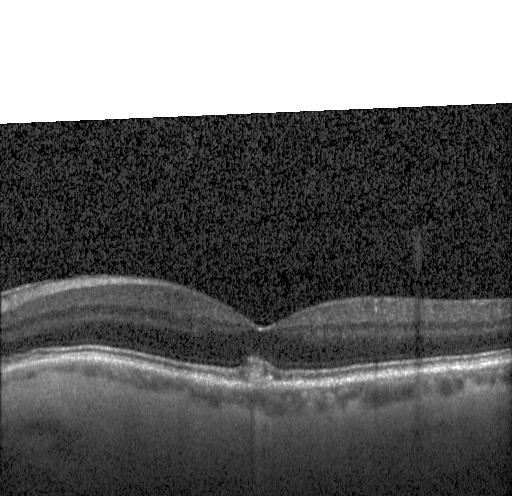

Optical coherence tomography B-scan. Assessment: drusen.